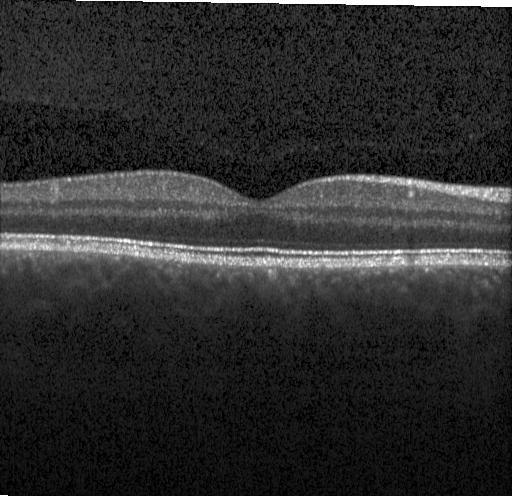
Diagnosis: no CNV, DME, or drusen.